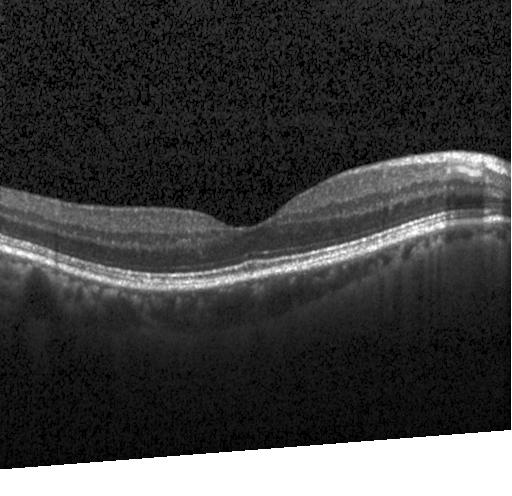
Centered on the fovea. SD-OCT. OCT line scan.
Finding: no choroidal neovascularization, no diabetic macular edema, and no drusen.